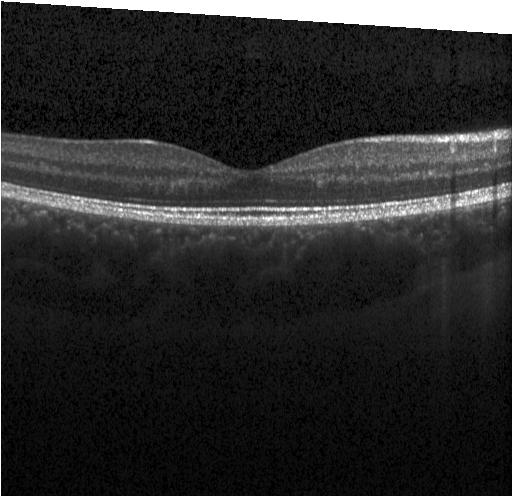
Optical coherence tomography scan.
Dx: neither CNV, DME, nor drusen.